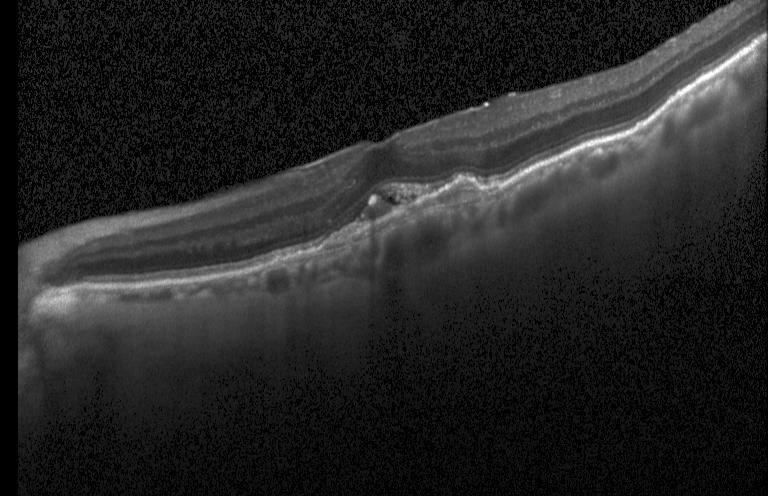
Horizontal scan through the fovea. Heidelberg Spectralis. OCT line scan. SD-OCT.
The scan shows choroidal neovascularization (CNV).